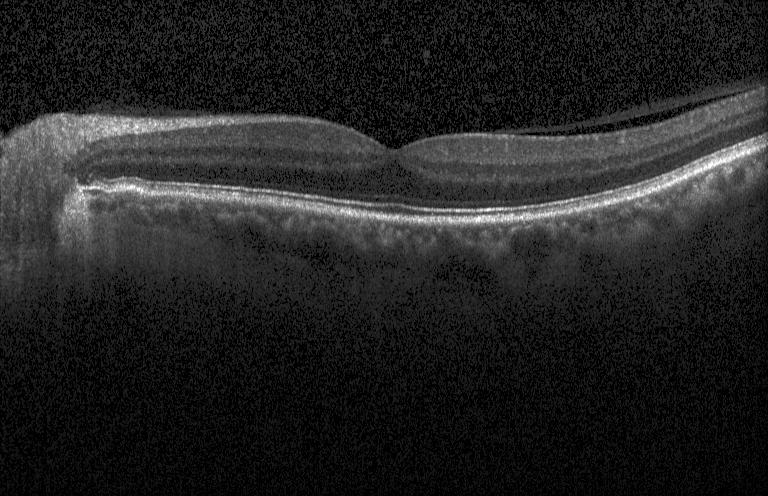

Acquired on a Heidelberg Spectralis. OCT B-scan — Impression: no evidence of choroidal neovascularization, diabetic macular edema, or drusen.